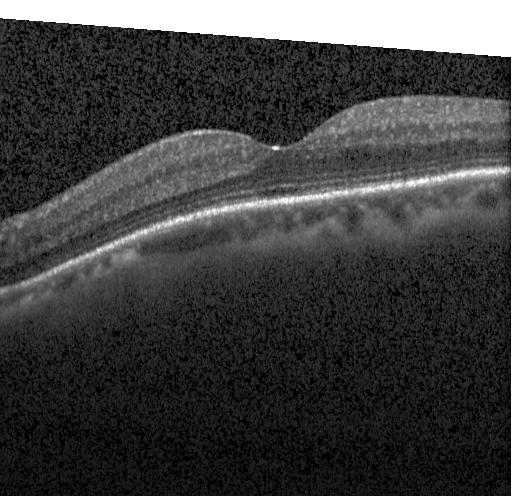

OCT B-scan — Macular OCT: neither choroidal neovascularization, diabetic macular edema, nor drusen.